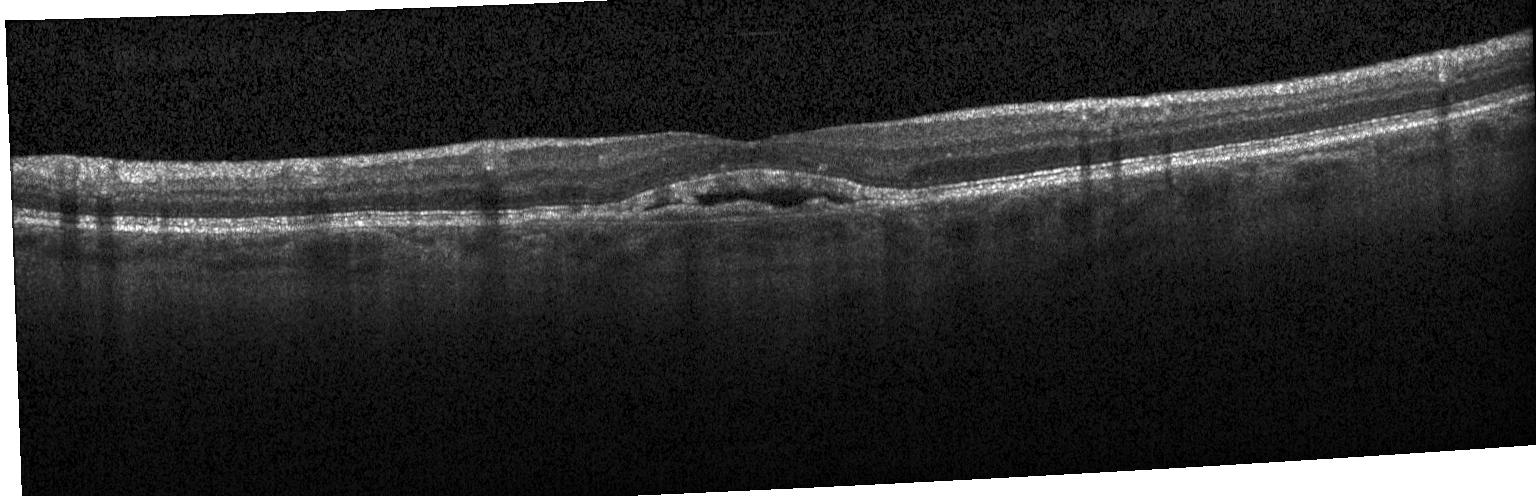 Spectral-domain OCT · retinal OCT cross-section.
Impression: choroidal neovascularization.